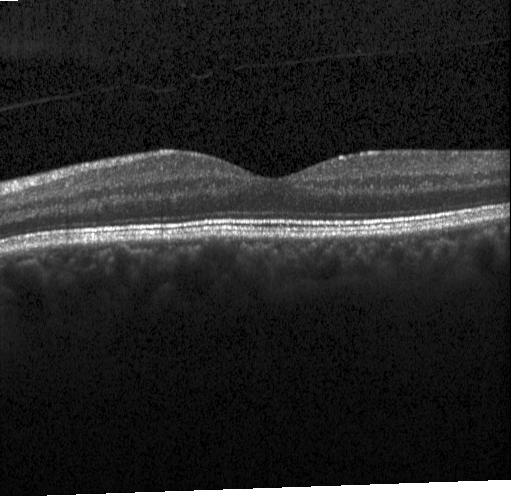

Through the macula; retinal OCT cross-section
This B-scan demonstrates no choroidal neovascularization, diabetic macular edema, or drusen.